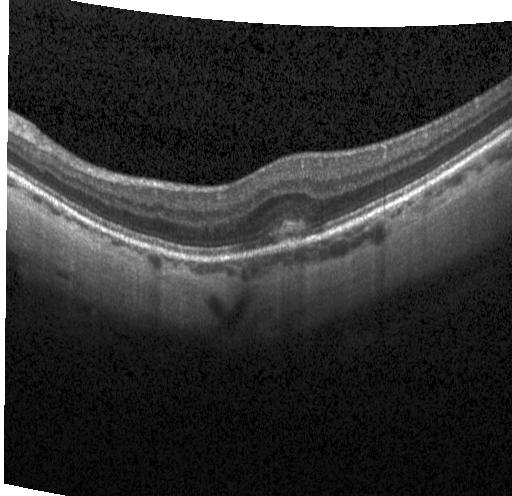 Optical coherence tomography B-scan, spectral-domain optical coherence tomography, Heidelberg Spectralis, macular scan. Diagnosis: choroidal neovascularization (CNV).